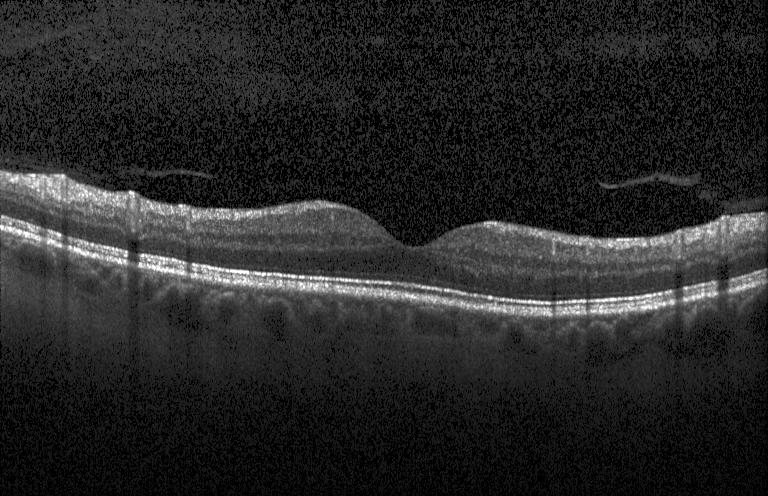
Optical coherence tomography B-scan, SD-OCT.
Diagnosis: no CNV, DME, or drusen.